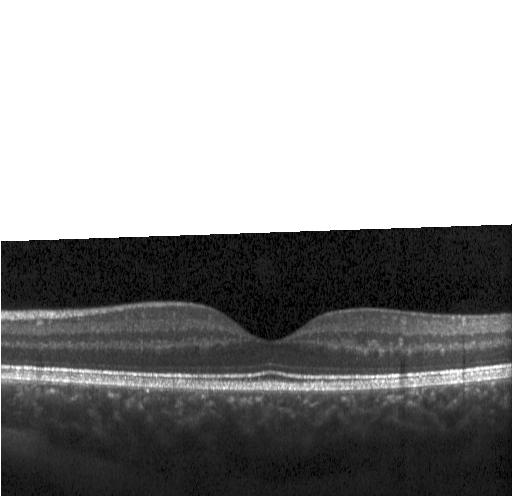
SD-OCT; retinal OCT B-scan — Assessment: no evidence of choroidal neovascularization, diabetic macular edema, or drusen.